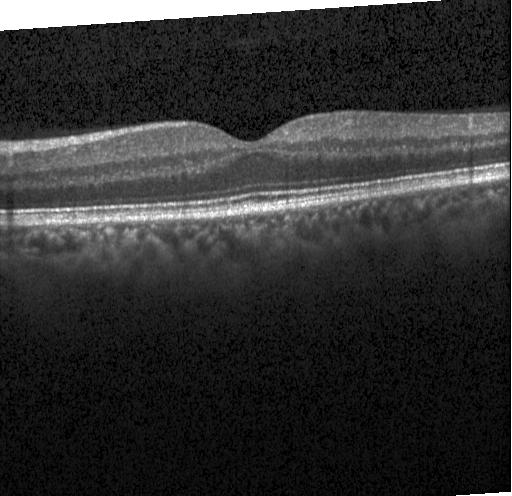
Finding: neither choroidal neovascularization, diabetic macular edema, nor drusen.